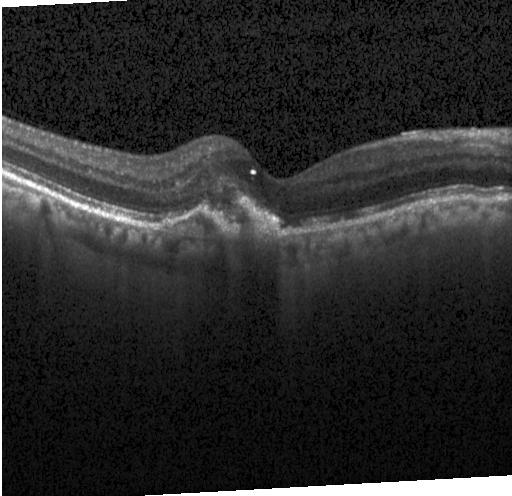 OCT line scan.
Assessment: a choroidal neovascular membrane.